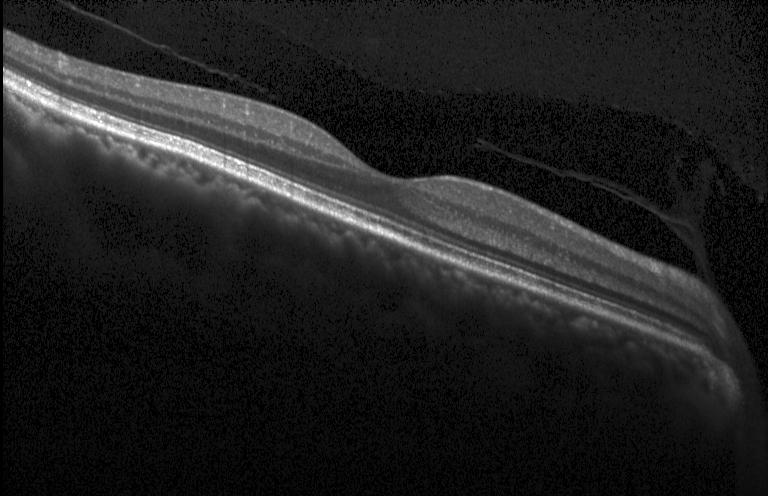 Macular scan, retinal OCT B-scan — No evidence of CNV, DME, or drusen.